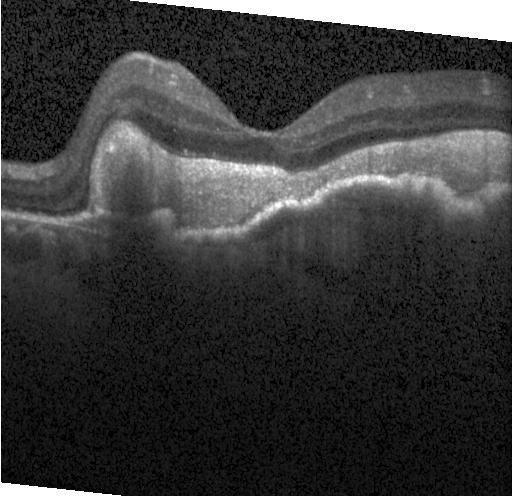

Retinal OCT cross-section.
Finding: a choroidal neovascular membrane.